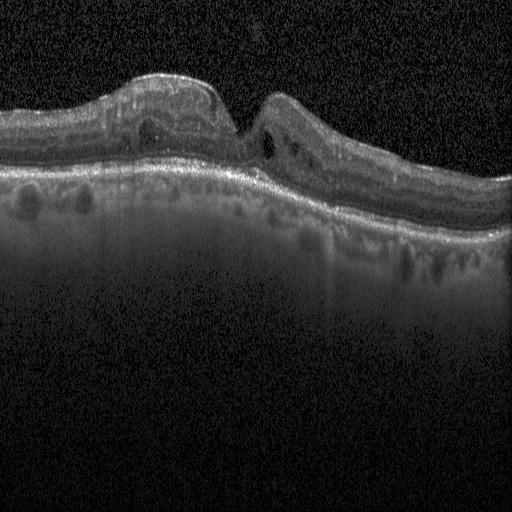 Diabetic macular edema (DME).